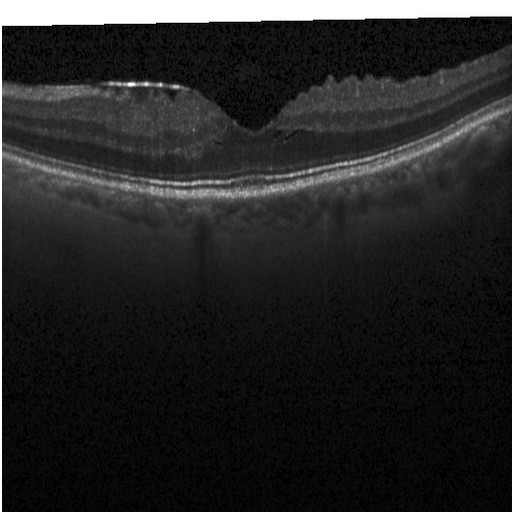 Spectral-domain OCT B-scan: DME.